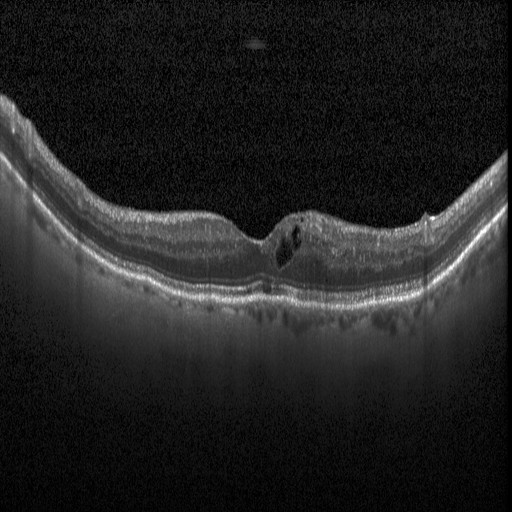

Diagnosis: DME.